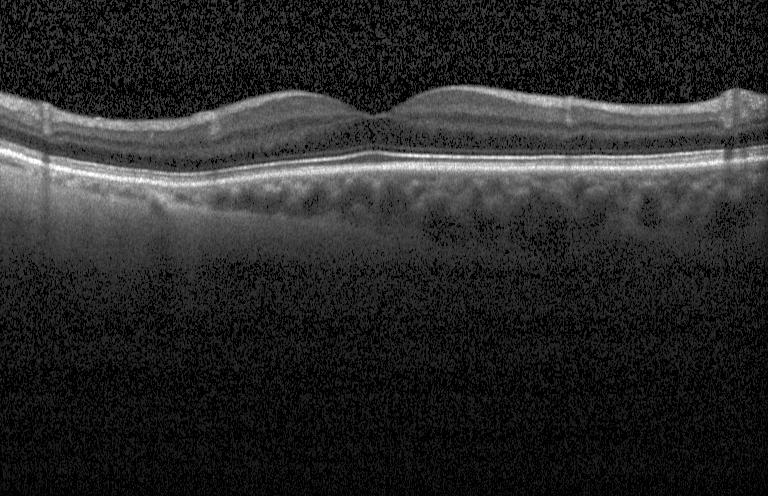
OCT finding: no choroidal neovascularization, diabetic macular edema, or drusen.